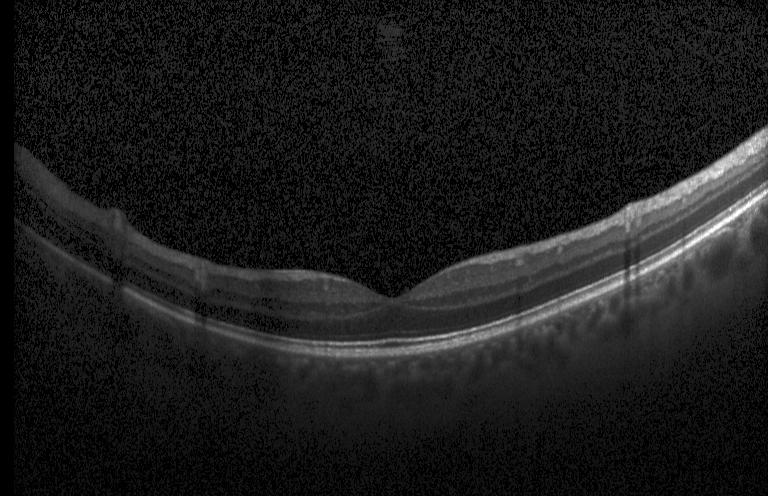 Finding: no choroidal neovascularization, diabetic macular edema, or drusen.